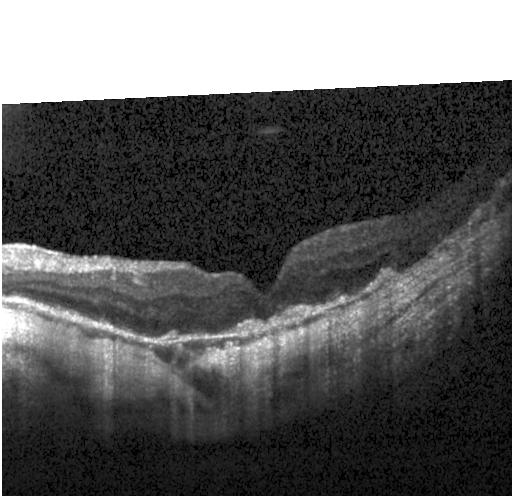
The scan shows CNV.